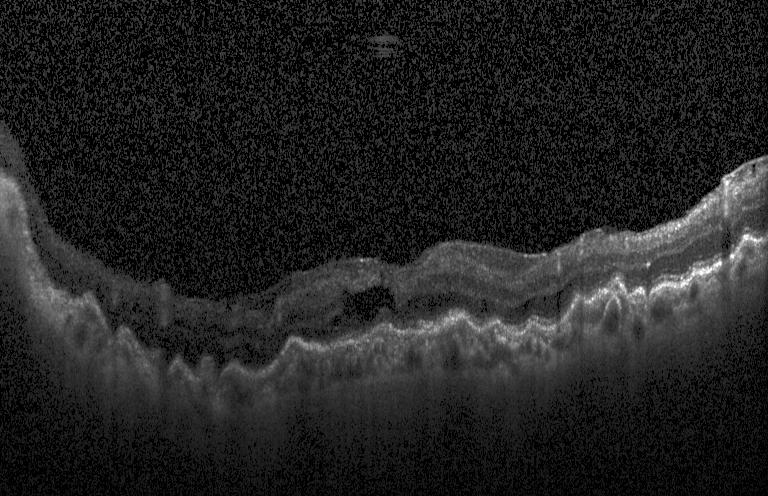
Acquired on a Heidelberg Spectralis. Spectral-domain optical coherence tomography. Retinal OCT B-scan. Centered on the fovea.
Impression: a choroidal neovascular membrane.